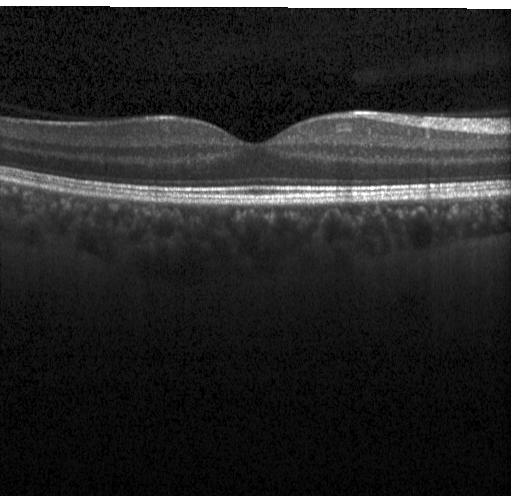
Acquired on a Heidelberg Spectralis; retinal OCT cross-section; centered on the fovea — Macular OCT: neither CNV, DME, nor drusen.